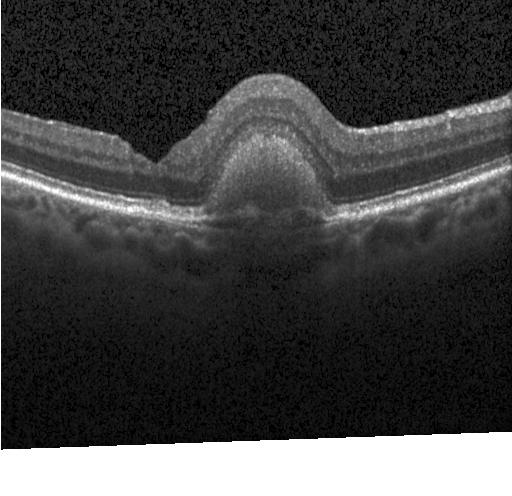

OCT line scan
The scan shows a choroidal neovascular membrane.